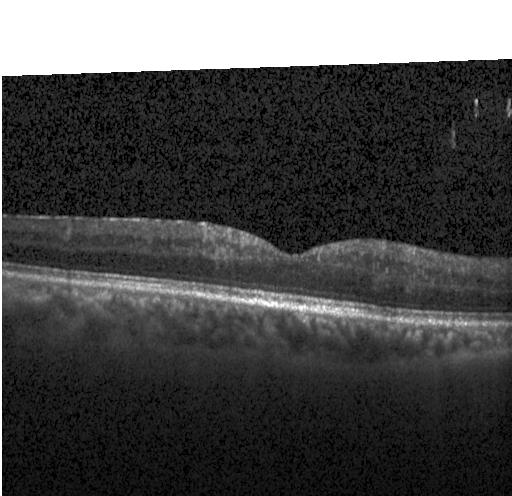
Retinal OCT cross-section showing no evidence of CNV, DME, or drusen.